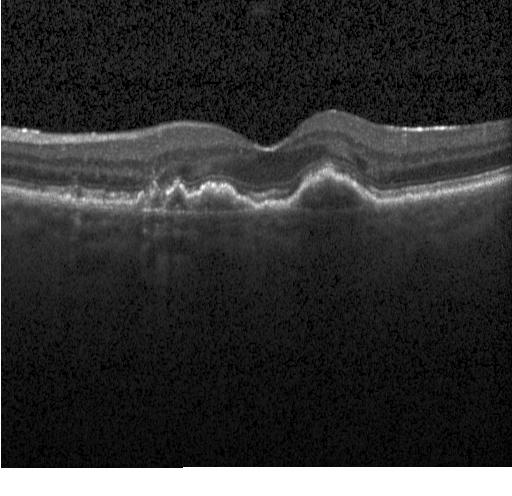

Optical coherence tomography B-scan — Macular OCT: a choroidal neovascular membrane.